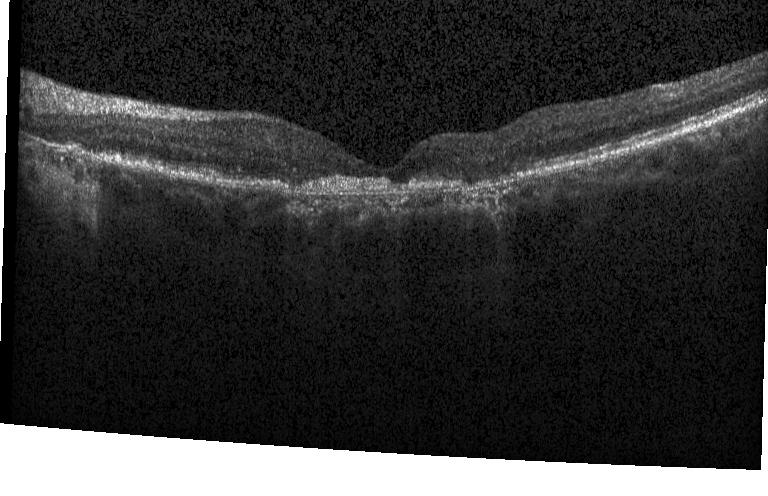
Diagnosis: a choroidal neovascular membrane.